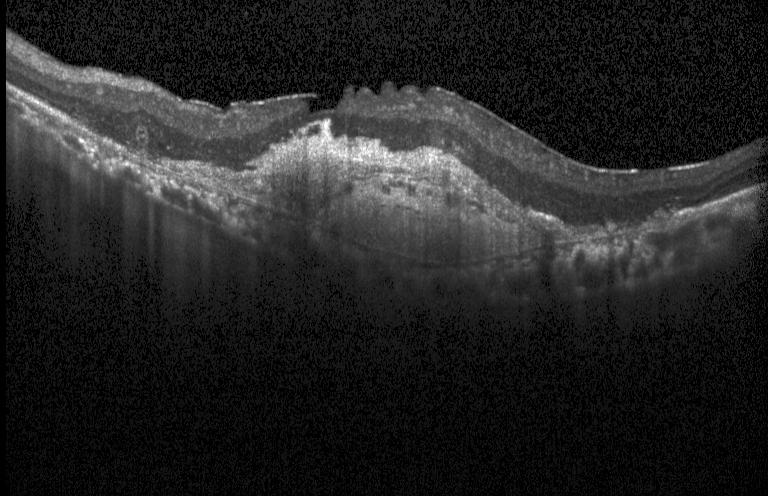
Spectral-domain OCT; through the macula; optical coherence tomography B-scan.
Assessment: CNV.